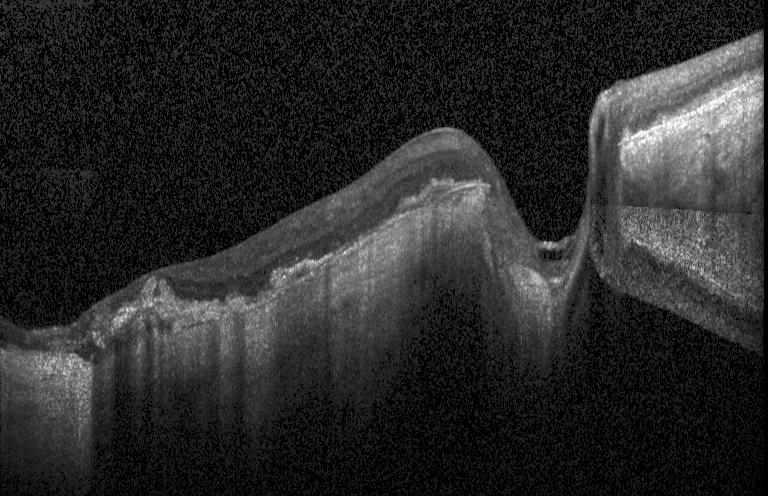
This B-scan demonstrates choroidal neovascularization.